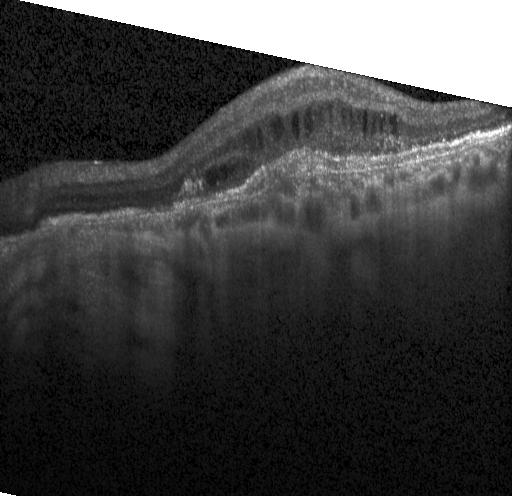 SD-OCT · OCT line scan
Impression: choroidal neovascularization.